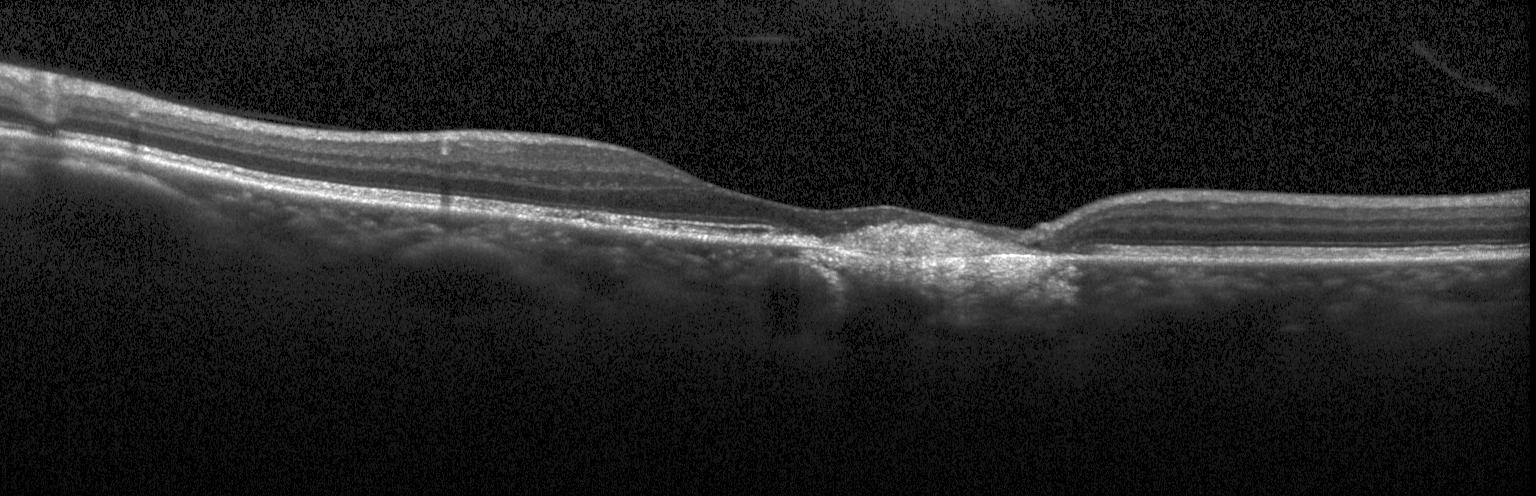 Retinal OCT B-scan
Macular OCT: choroidal neovascularization (CNV).